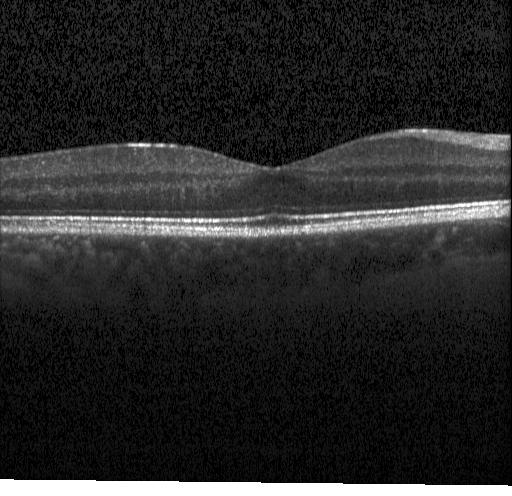

Spectral-domain OCT B-scan: no choroidal neovascularization, no diabetic macular edema, and no drusen.